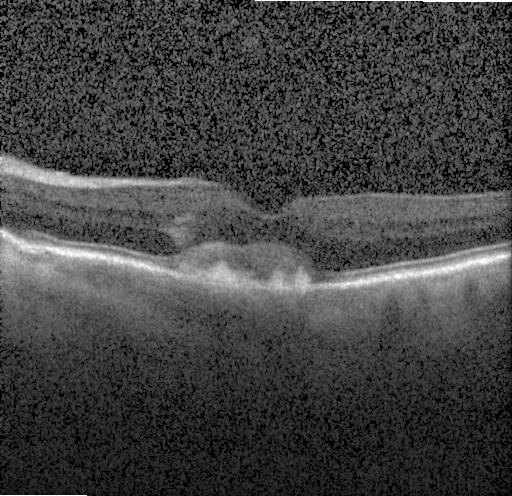 Optical coherence tomography B-scan. Instrument: Heidelberg Spectralis
Finding: choroidal neovascularization.